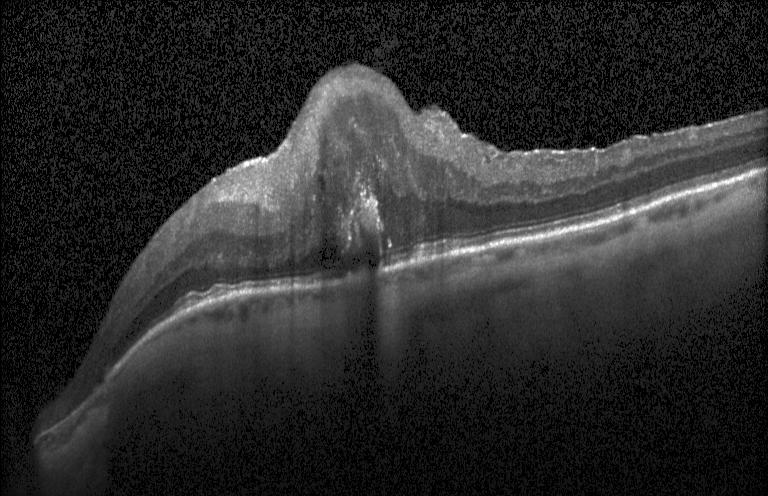 Instrument: Heidelberg Spectralis. Spectral-domain optical coherence tomography. Optical coherence tomography B-scan. Through the macula
Finding: choroidal neovascularization.